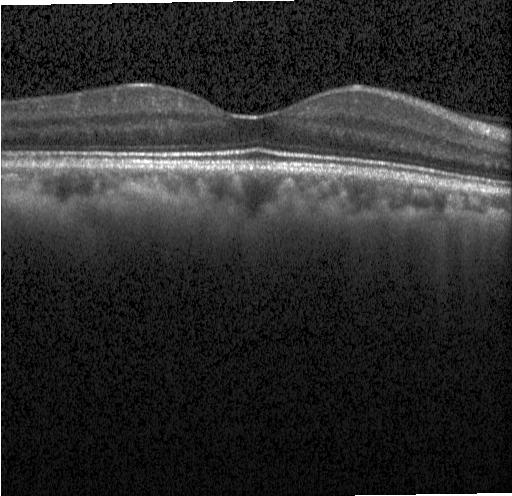

Acquired on a Heidelberg Spectralis, SD-OCT, through the macula, retinal OCT B-scan — No CNV, DME, or drusen.